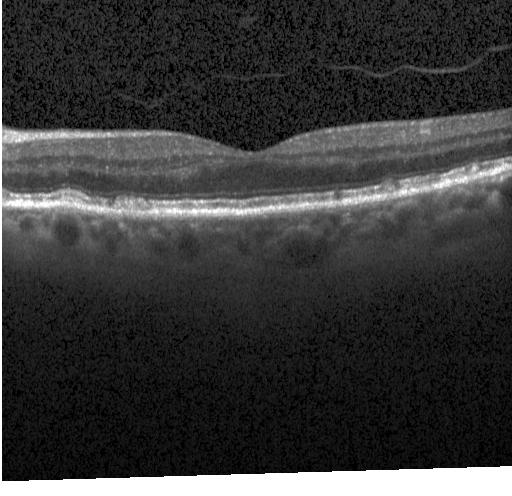 Macular OCT demonstrating drusen.